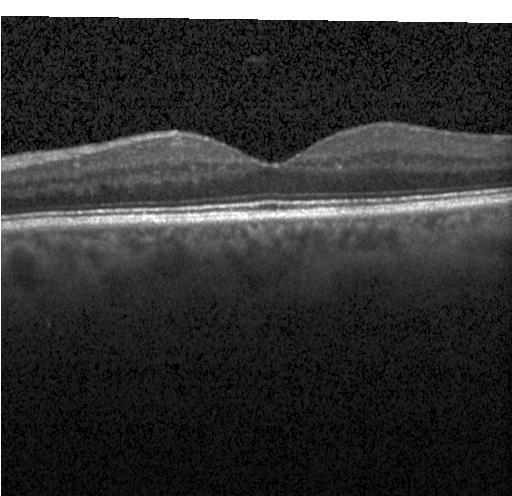

Retinal OCT B-scan; through the macula; acquired on a Heidelberg Spectralis.
No evidence of choroidal neovascularization, diabetic macular edema, or drusen.